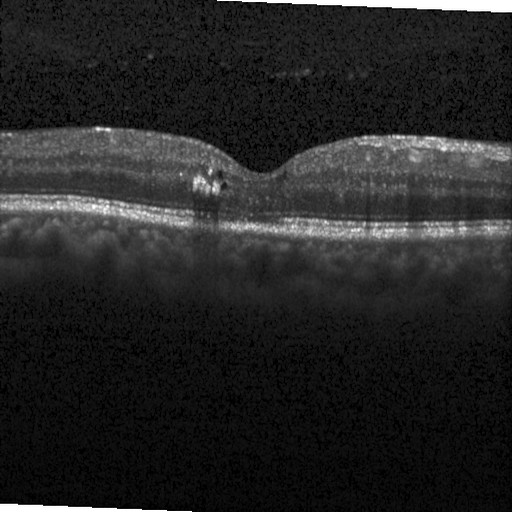 Optical coherence tomography scan · Heidelberg Spectralis OCT system · SD-OCT
Impression: diabetic macular edema (DME).